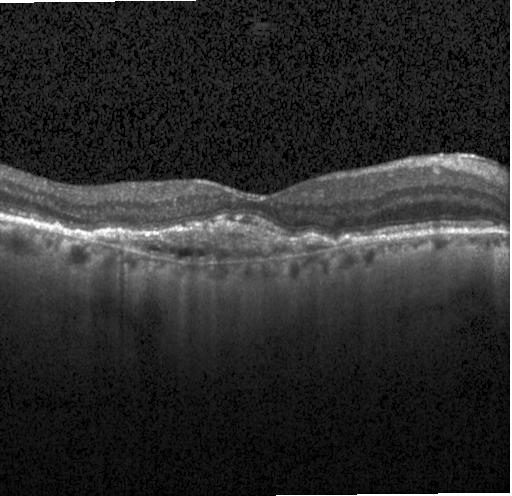
Diagnosis: choroidal neovascularization (CNV).